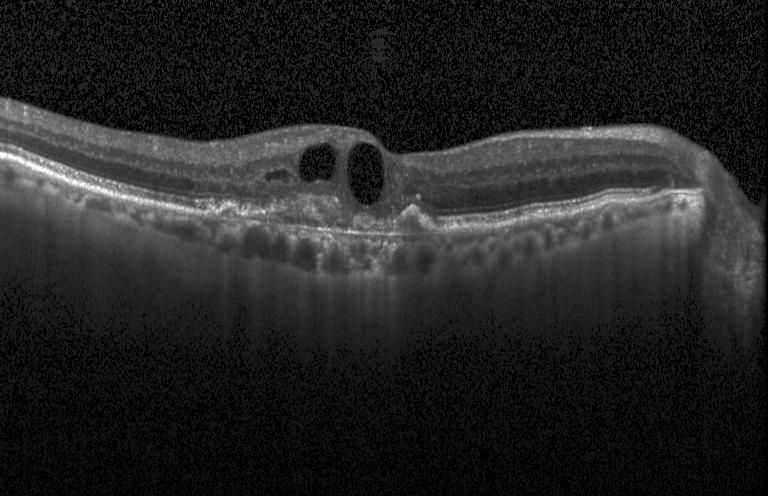 Horizontal scan through the fovea, Heidelberg Spectralis, OCT line scan
Finding: a choroidal neovascular membrane.